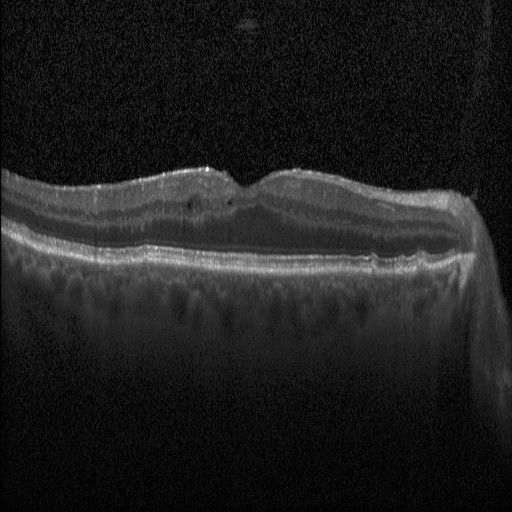 Instrument: Heidelberg Spectralis · through the macula · retinal OCT cross-section
The scan shows DME.